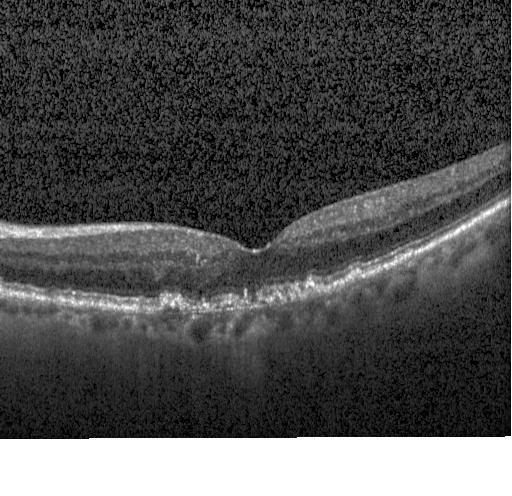
Retinal OCT cross-section; Heidelberg Spectralis; SD-OCT; centered on the fovea — This B-scan demonstrates multiple drusen.